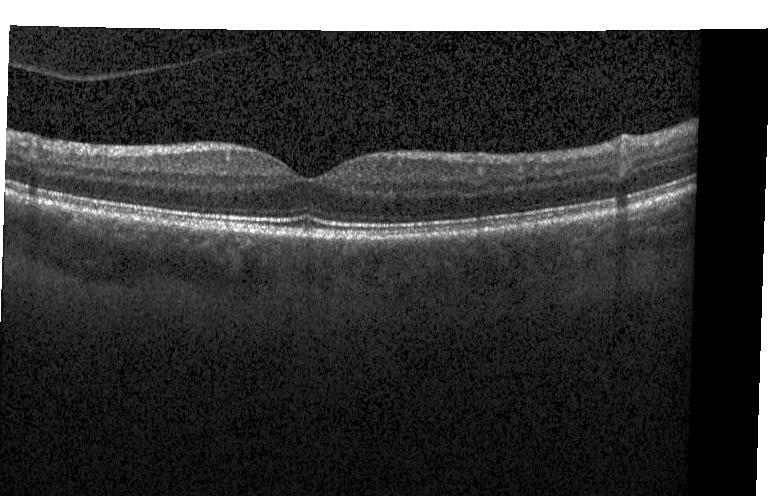

Dx: no choroidal neovascularization, no diabetic macular edema, and no drusen.